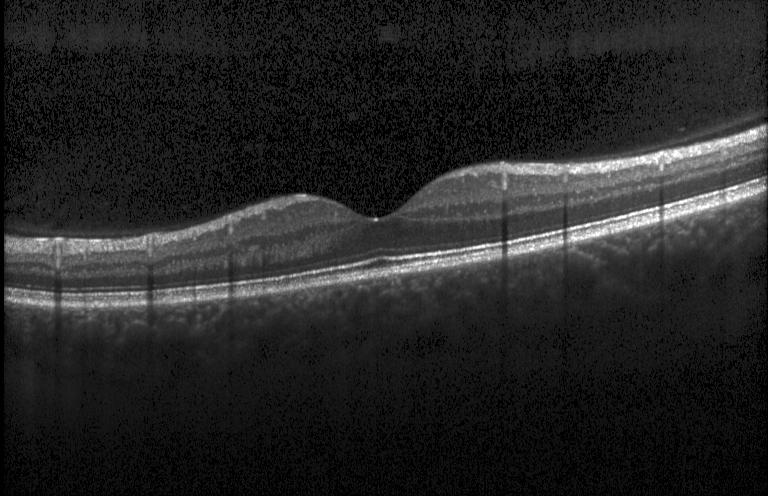
Optical coherence tomography B-scan. The scan shows neither choroidal neovascularization, diabetic macular edema, nor drusen.